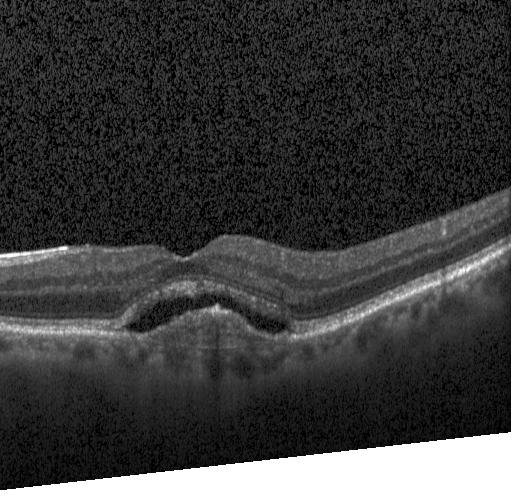 Optical coherence tomography scan. Heidelberg Spectralis OCT system. Horizontal scan through the fovea — Diagnosis: choroidal neovascularization.